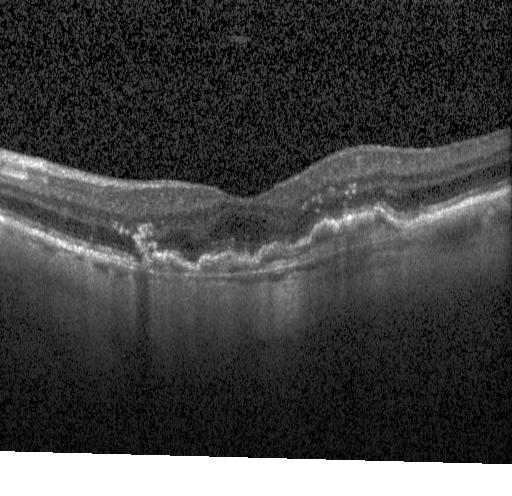

Heidelberg Spectralis; horizontal scan through the fovea; optical coherence tomography scan — Assessment: choroidal neovascularization.